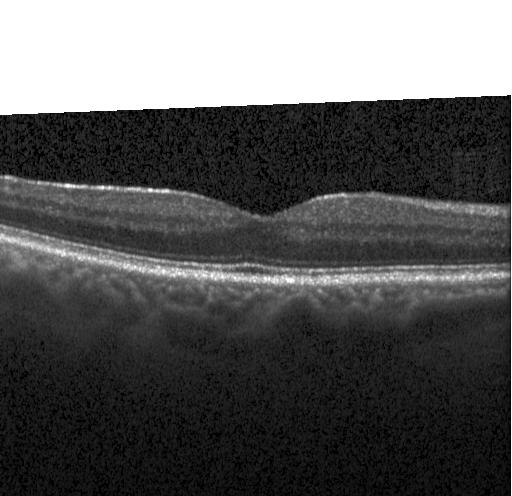

Optical coherence tomography B-scan
Diagnosis: no choroidal neovascularization, diabetic macular edema, or drusen.